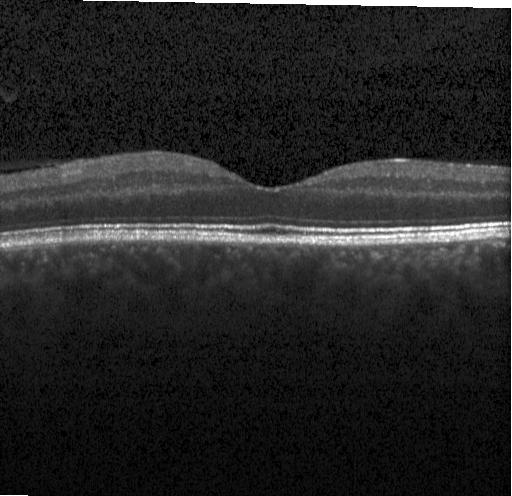

Macular OCT demonstrating neither choroidal neovascularization, diabetic macular edema, nor drusen.